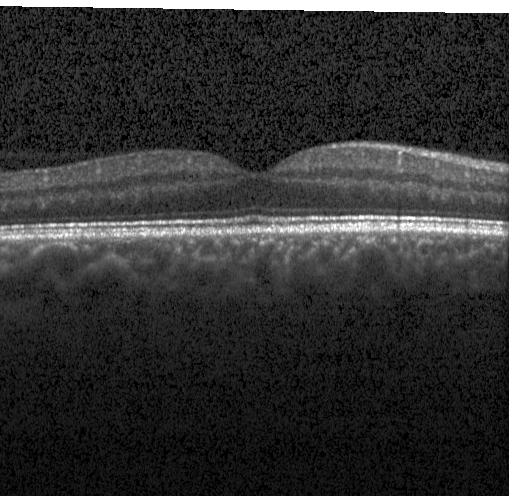

Macular scan; retinal OCT B-scan
Macular OCT: no evidence of choroidal neovascularization, diabetic macular edema, or drusen.